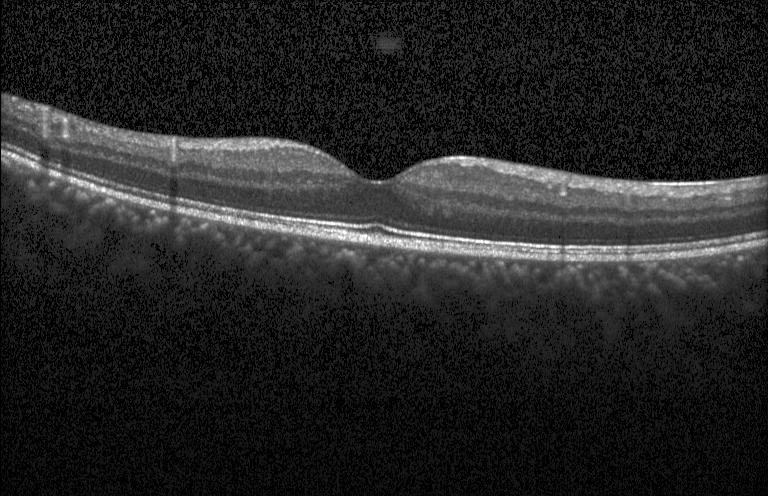

The scan shows neither choroidal neovascularization, diabetic macular edema, nor drusen.